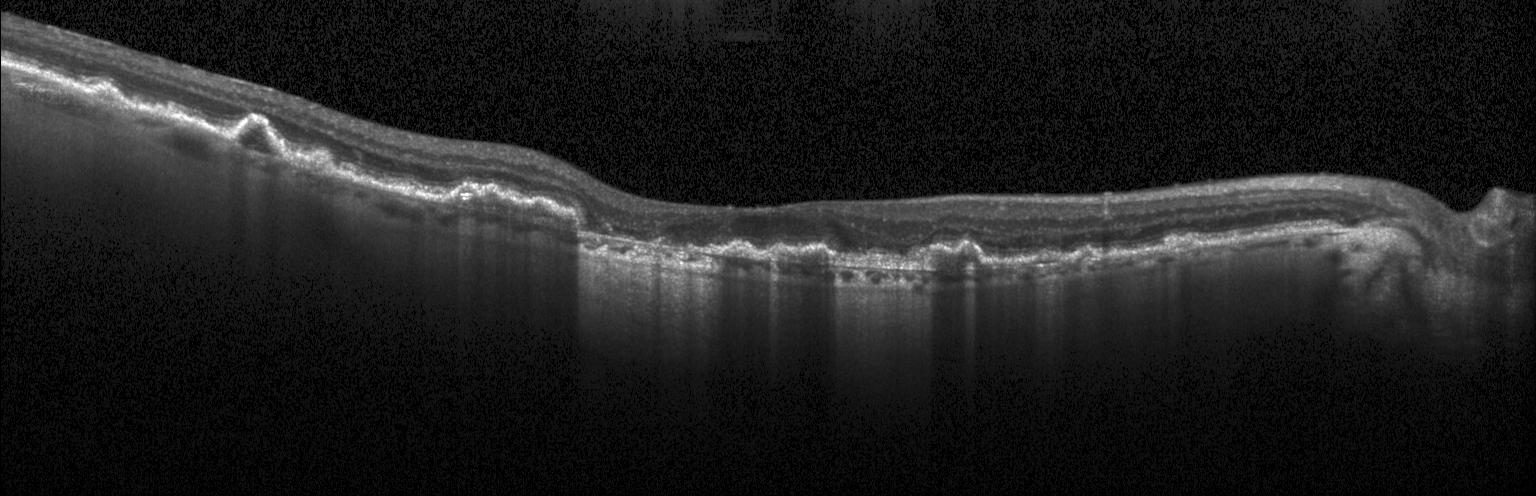
Spectral-domain optical coherence tomography; retinal OCT B-scan; instrument: Heidelberg Spectralis.
This B-scan demonstrates choroidal neovascularization (CNV).